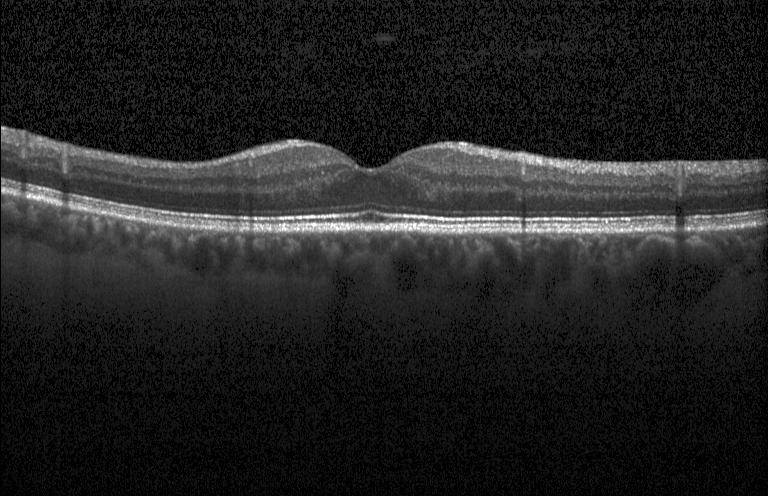
OCT B-scan showing no CNV, no DME, and no drusen.